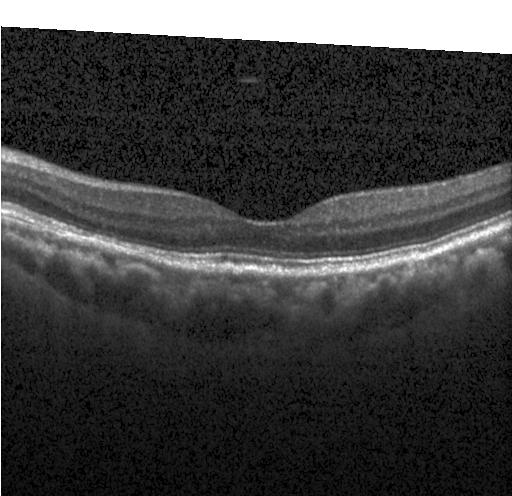
Diagnosis: neither choroidal neovascularization, diabetic macular edema, nor drusen.